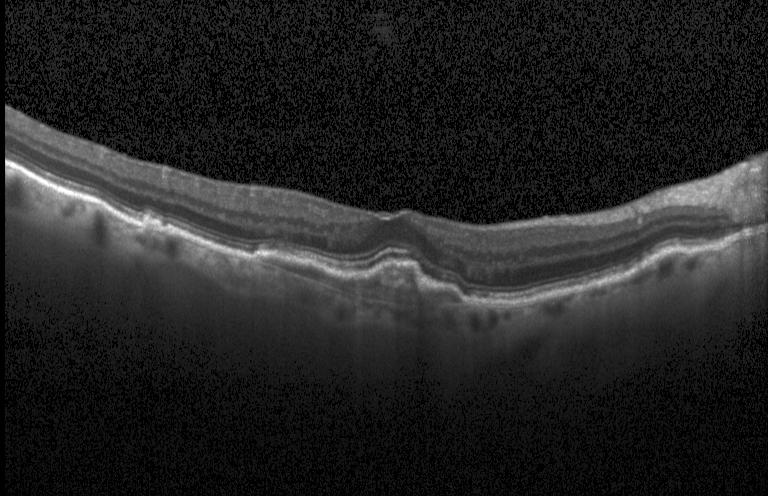 Optical coherence tomography scan.
OCT finding: choroidal neovascularization.